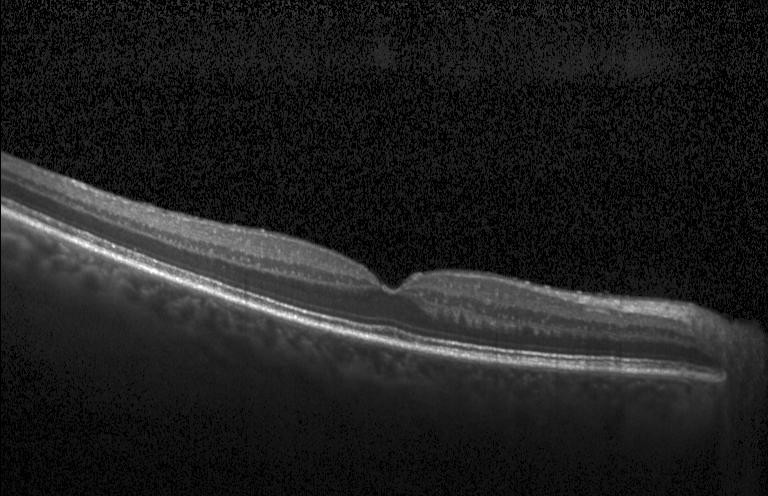
OCT line scan
Finding: neither CNV, DME, nor drusen.